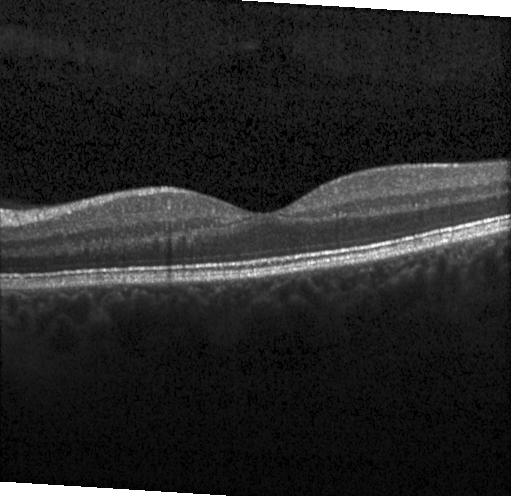

OCT B-scan. Diagnosis: no CNV, DME, or drusen.